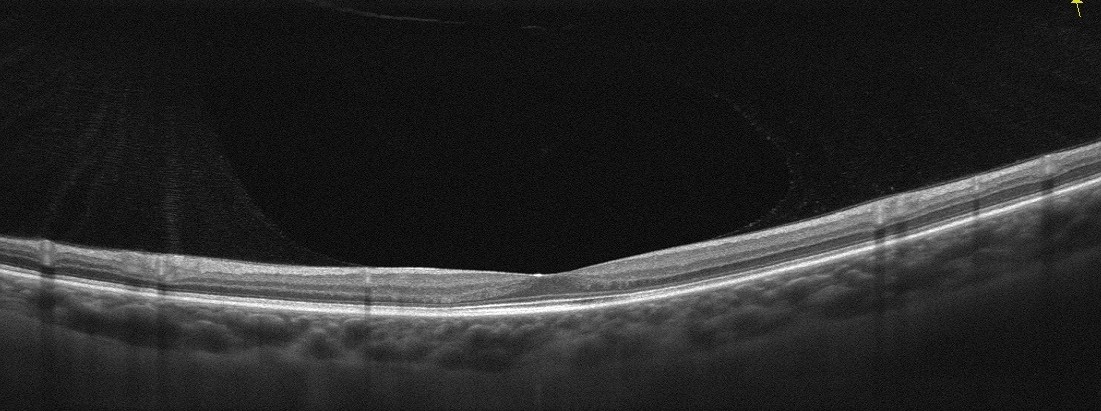

Macular OCT demonstrating absence of AMD, DME, ERM, RAO, RVO, and vitreomacular interface disease.